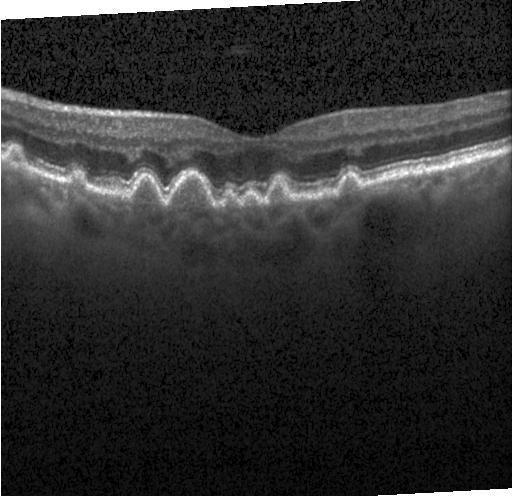 Acquired on a Heidelberg Spectralis. Centered on the fovea. Spectral-domain OCT. Optical coherence tomography scan.
This B-scan demonstrates multiple drusen.